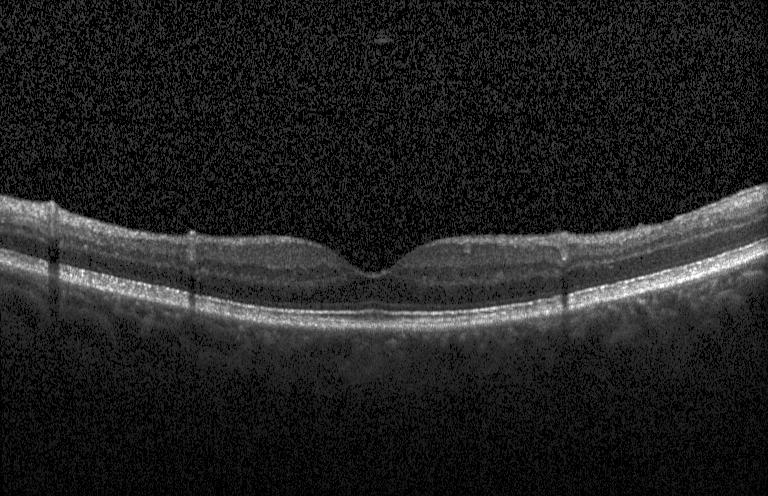
Centered on the fovea; OCT B-scan; Heidelberg Spectralis OCT system.
Impression: no evidence of choroidal neovascularization, diabetic macular edema, or drusen.